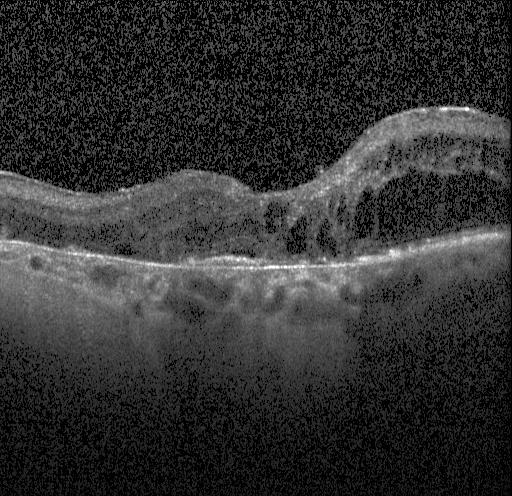
Dx: CNV.